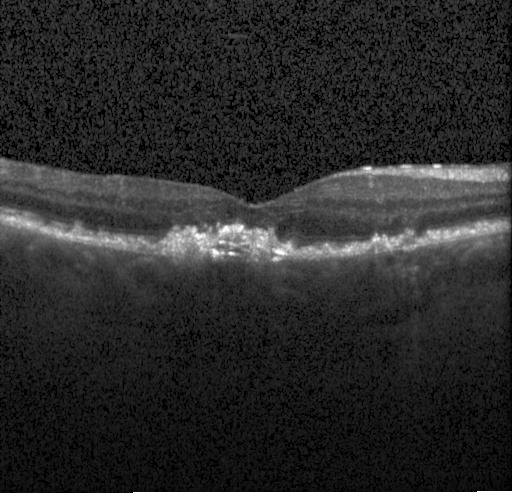 OCT scan showing choroidal neovascularization.